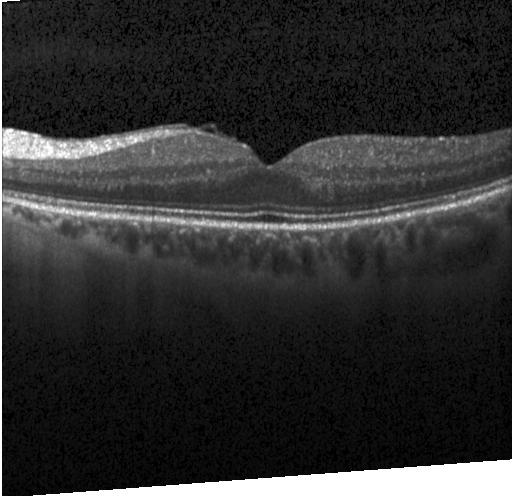 Macular OCT demonstrating no evidence of choroidal neovascularization, diabetic macular edema, or drusen.